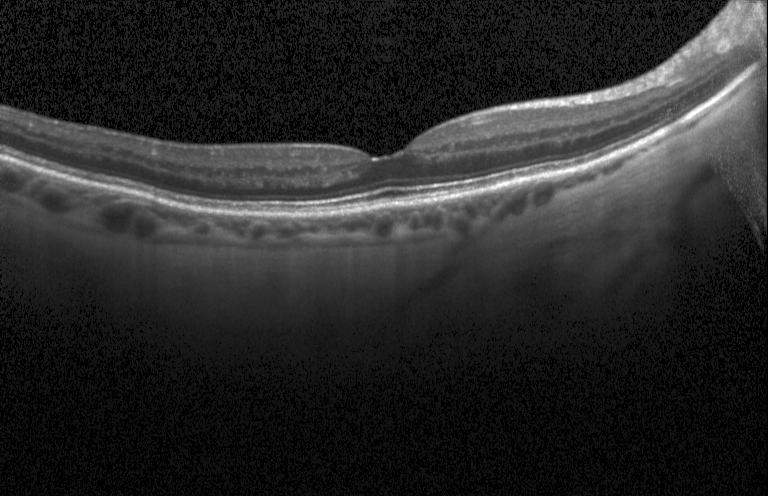
Optical coherence tomography B-scan, centered on the fovea, spectral-domain optical coherence tomography, acquired on a Heidelberg Spectralis. Finding: neither choroidal neovascularization, diabetic macular edema, nor drusen.